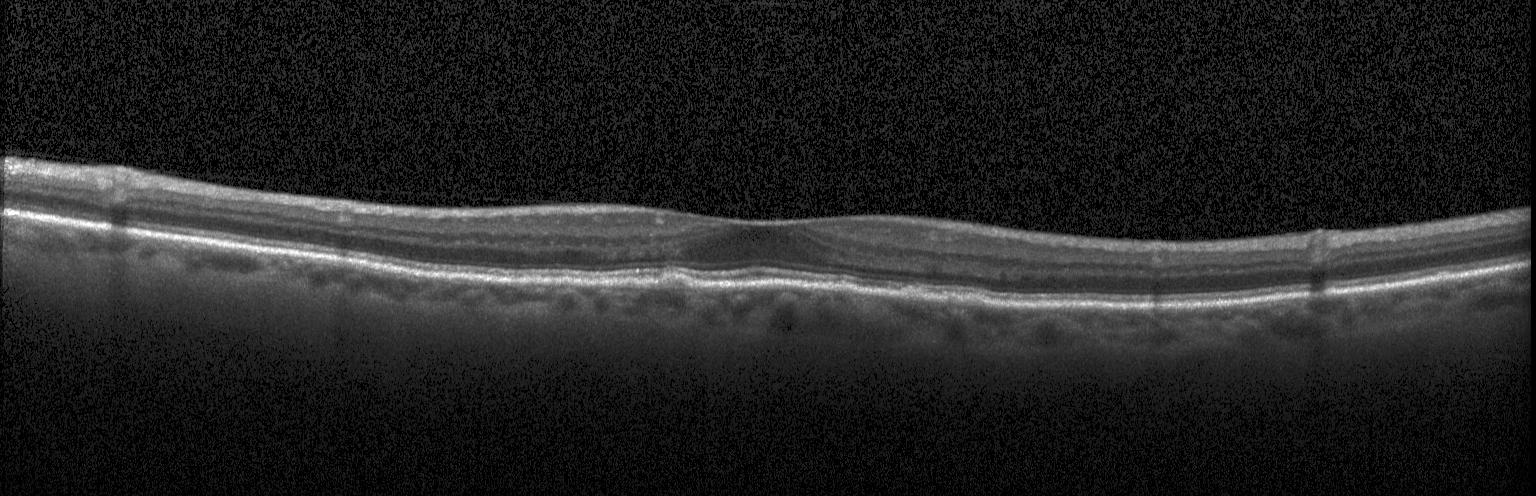
Macular OCT: multiple drusen.